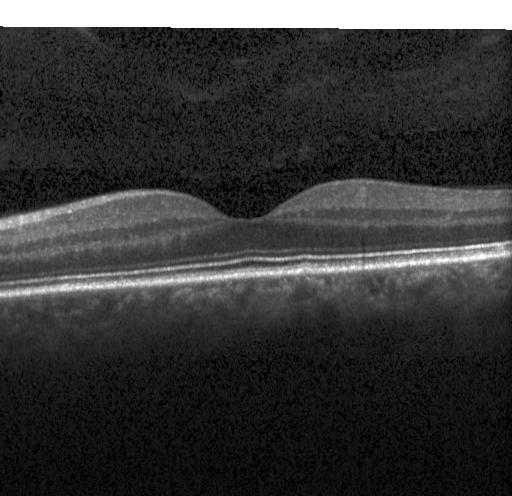 Spectral-domain OCT B-scan: no evidence of choroidal neovascularization, diabetic macular edema, or drusen.